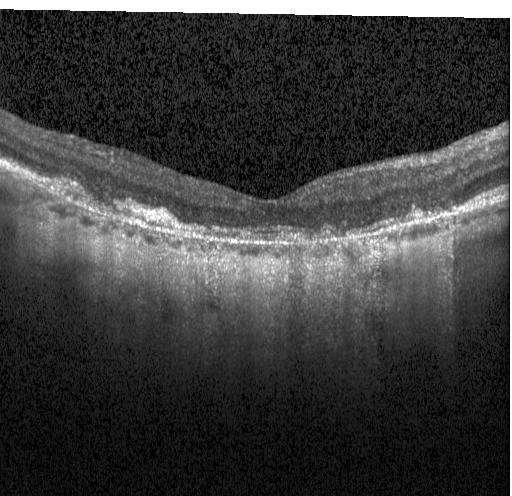

Retinal OCT cross-section showing a choroidal neovascular membrane.